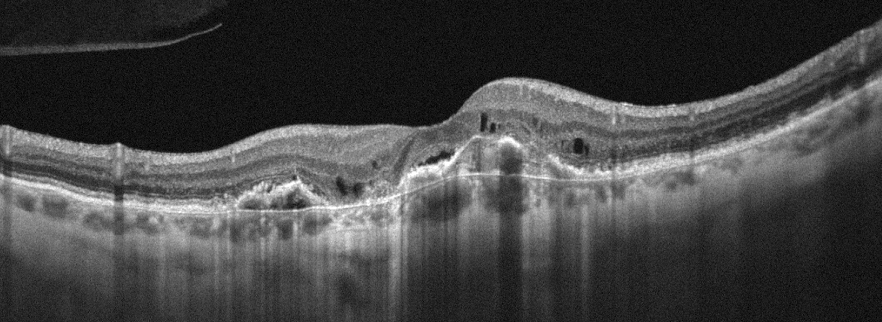

Impression: age-related macular degeneration (AMD).